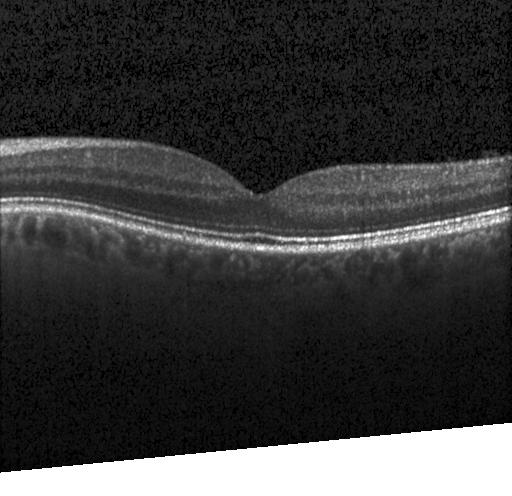

Macular OCT: no CNV, DME, or drusen.